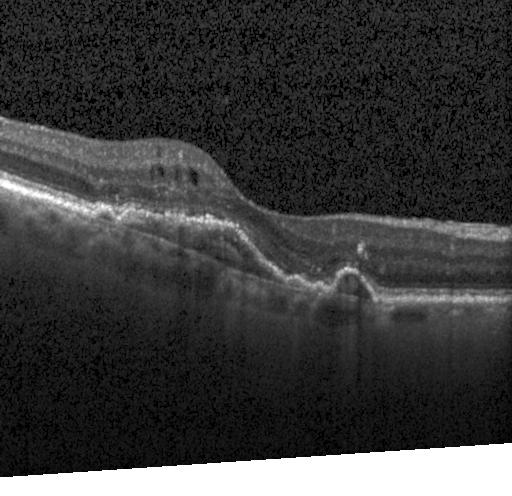

Horizontal scan through the fovea; retinal OCT B-scan; Heidelberg Spectralis OCT system; spectral-domain OCT
Assessment: a choroidal neovascular membrane.